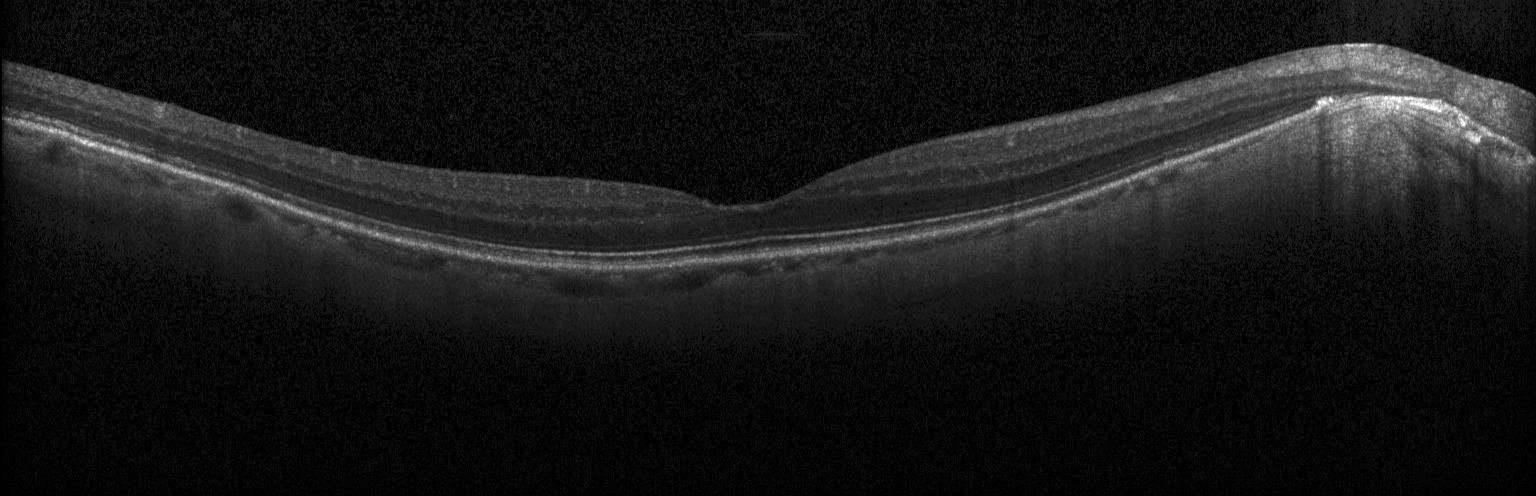 Spectral-domain optical coherence tomography; Heidelberg Spectralis; optical coherence tomography scan
Finding: no choroidal neovascularization, no diabetic macular edema, and no drusen.